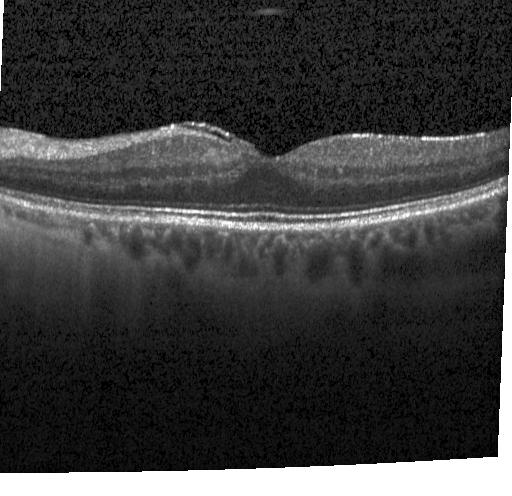

Impression: no choroidal neovascularization, diabetic macular edema, or drusen.